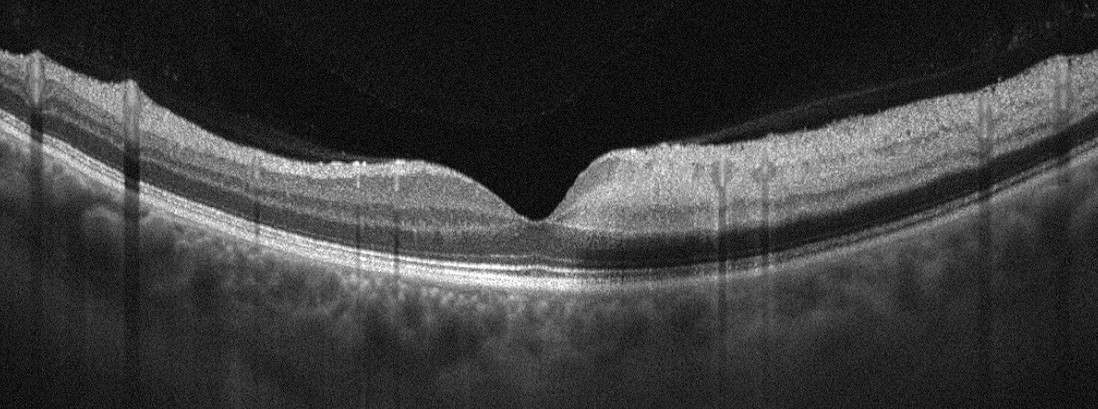

OCT B-scan. Assessment: retinal artery occlusion.